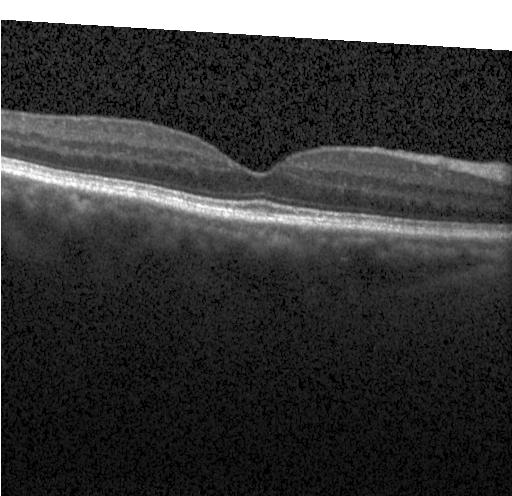 The scan shows no choroidal neovascularization, diabetic macular edema, or drusen.